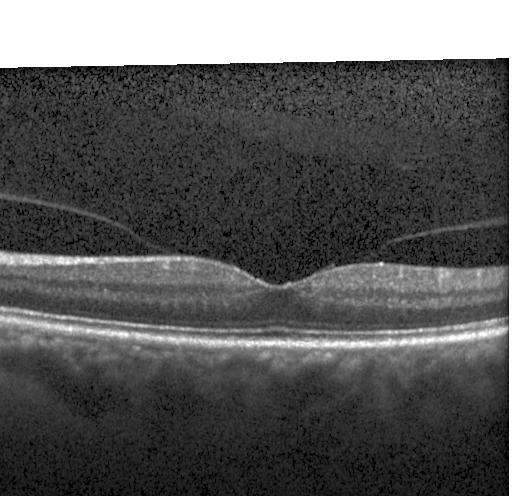 Retinal OCT B-scan · Heidelberg Spectralis OCT system · centered on the fovea · spectral-domain OCT.
Impression: no evidence of choroidal neovascularization, diabetic macular edema, or drusen.